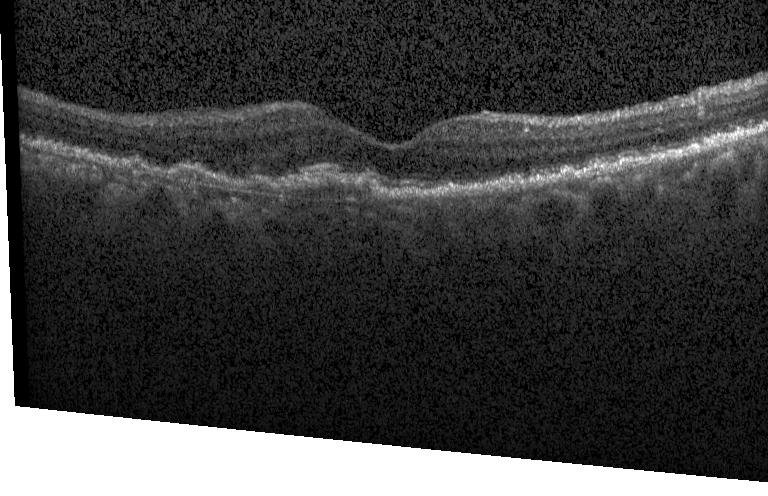

Optical coherence tomography B-scan.
The scan shows CNV.